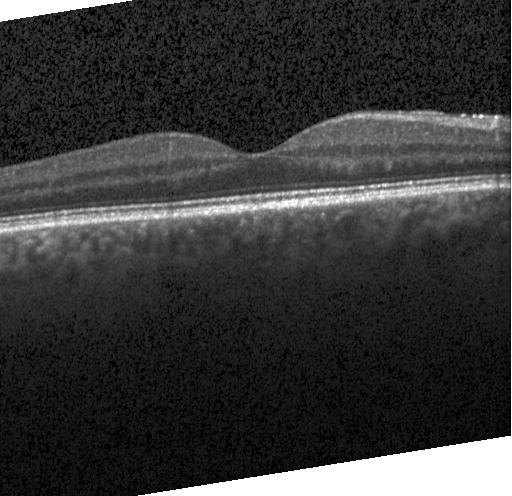
Heidelberg Spectralis. Fovea-centered. Optical coherence tomography scan.
Diagnosis: neither CNV, DME, nor drusen.